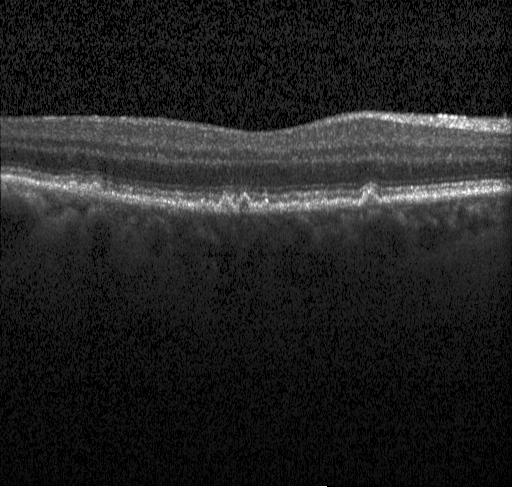
Multiple drusen.